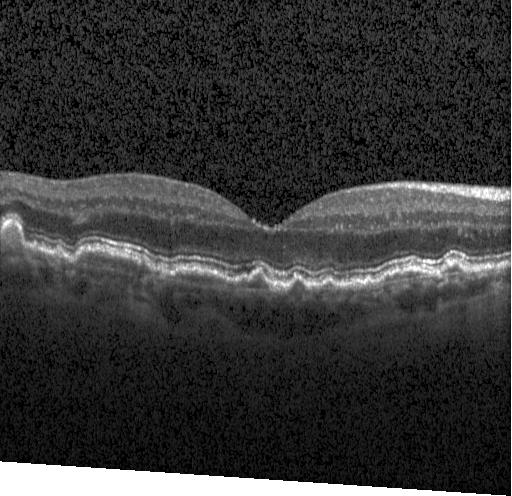

OCT B-scan showing drusen.